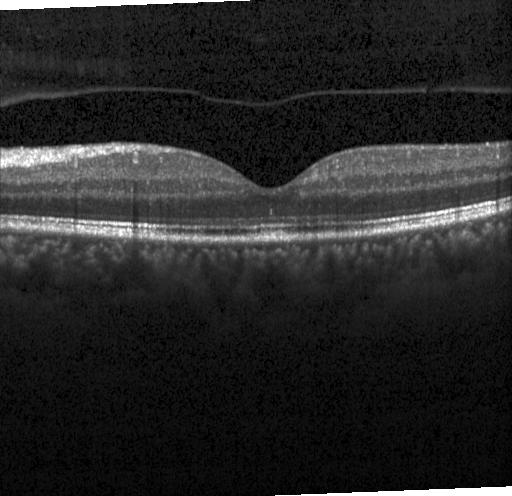 Heidelberg Spectralis OCT system. OCT B-scan
No evidence of choroidal neovascularization, diabetic macular edema, or drusen.